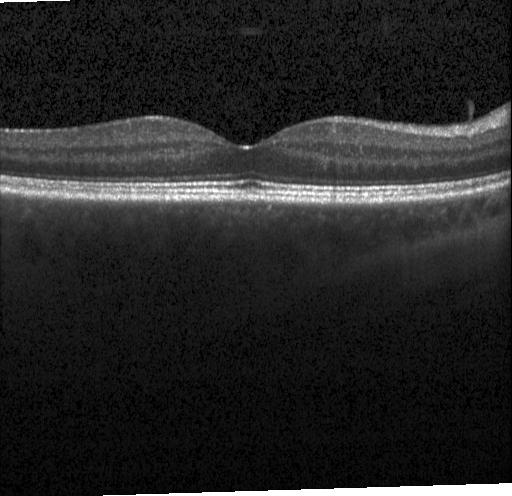 Macular scan; optical coherence tomography B-scan.
Impression: no choroidal neovascularization, diabetic macular edema, or drusen.